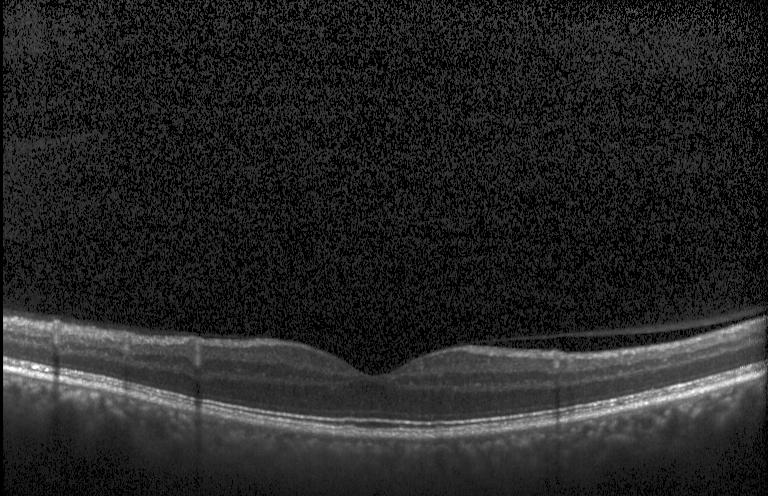 OCT B-scan
OCT finding: no CNV, no DME, and no drusen.